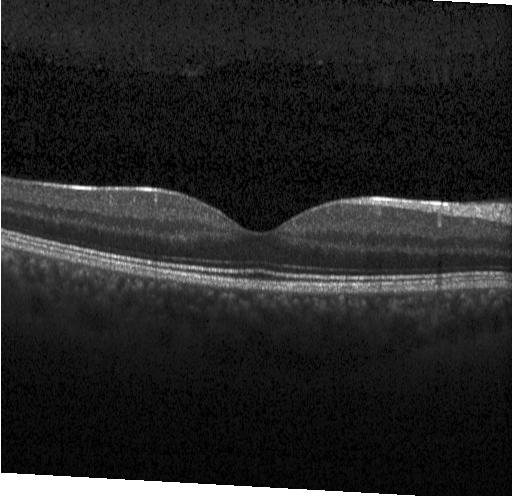

Diagnosis: no evidence of CNV, DME, or drusen.